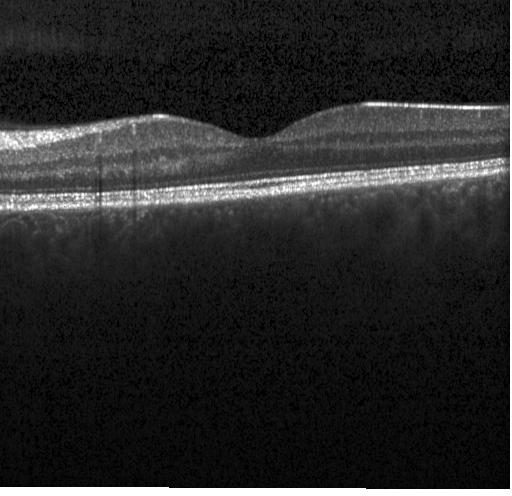

Retinal OCT cross-section, SD-OCT, Heidelberg Spectralis, fovea-centered.
Macular OCT: no choroidal neovascularization, diabetic macular edema, or drusen.